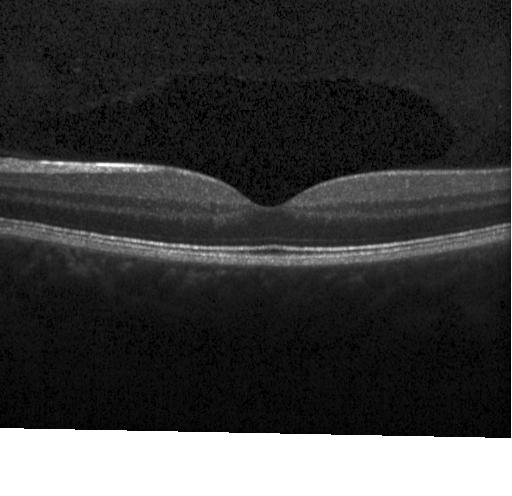
Macular OCT demonstrating no choroidal neovascularization, no diabetic macular edema, and no drusen.